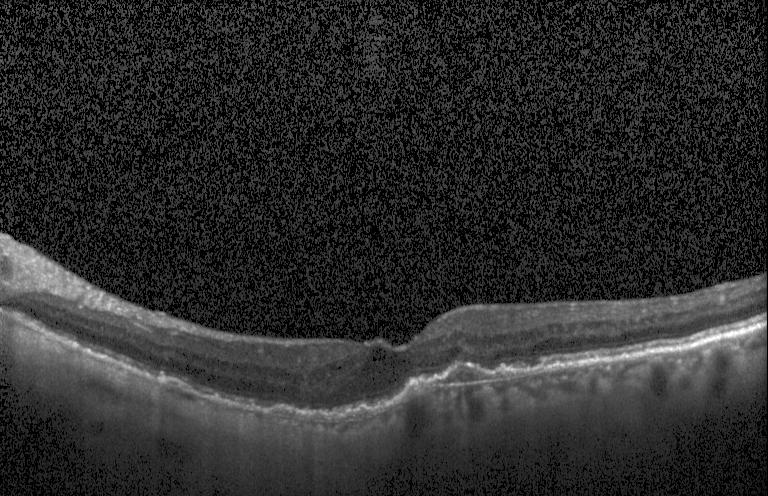
Diagnosis: CNV.